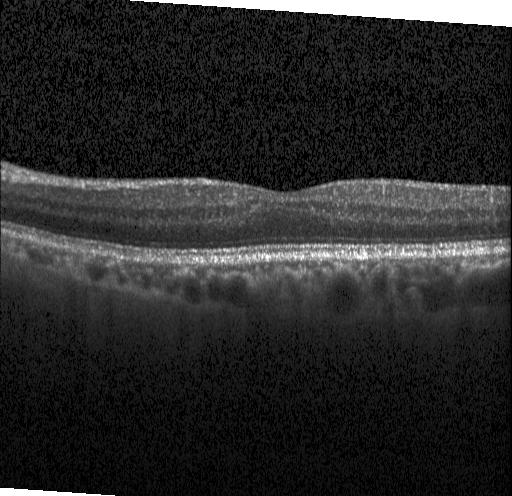
OCT finding: no evidence of CNV, DME, or drusen.